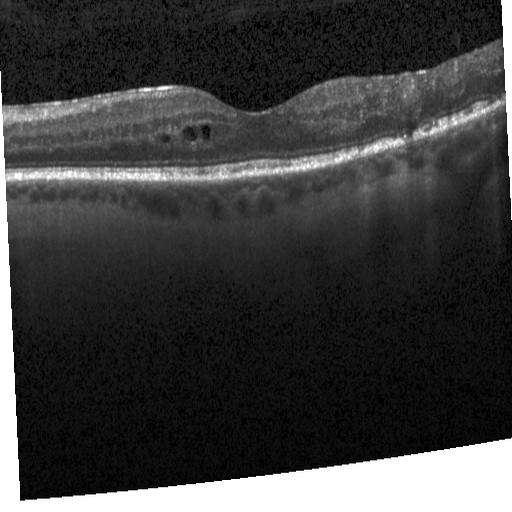

SD-OCT · fovea-centered · retinal OCT cross-section · Heidelberg Spectralis. Impression: diabetic macular edema (DME).